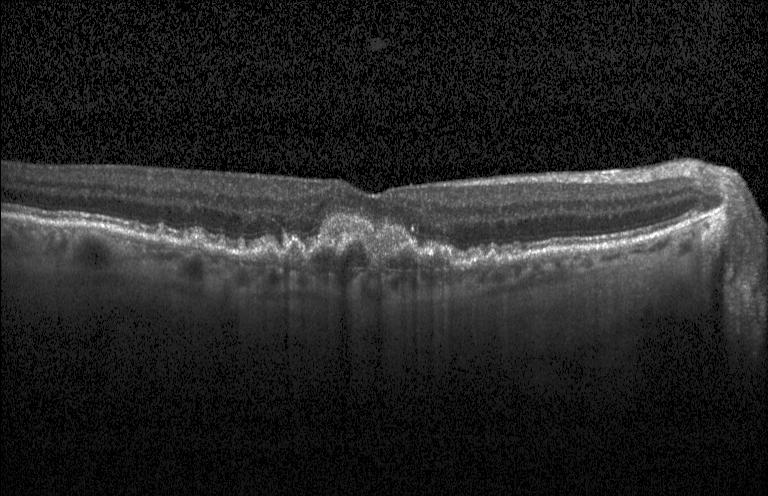
Assessment: CNV.